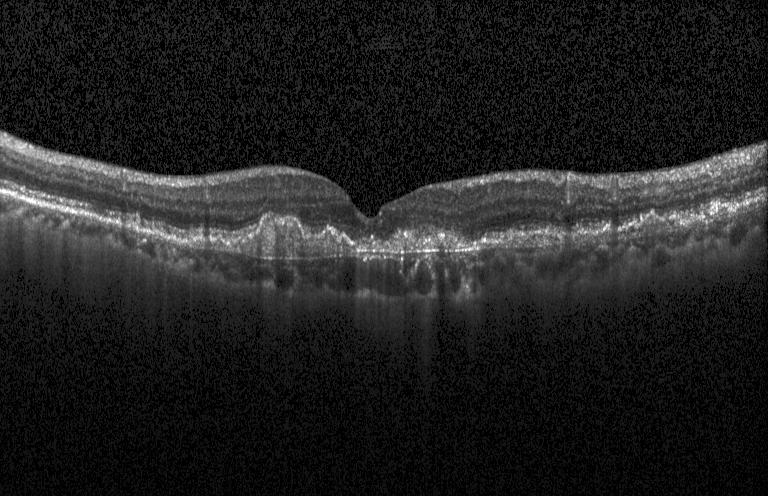 Optical coherence tomography scan · spectral-domain OCT · macular scan
Macular OCT: choroidal neovascularization (CNV).